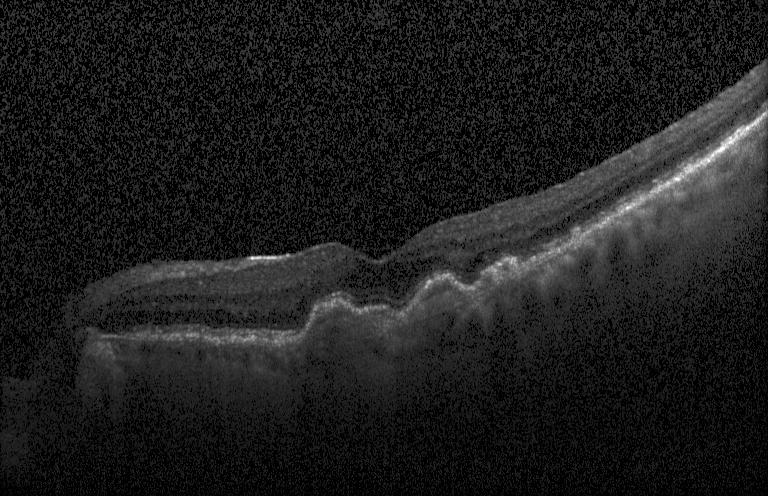

SD-OCT, OCT B-scan.
Assessment: a choroidal neovascular membrane.